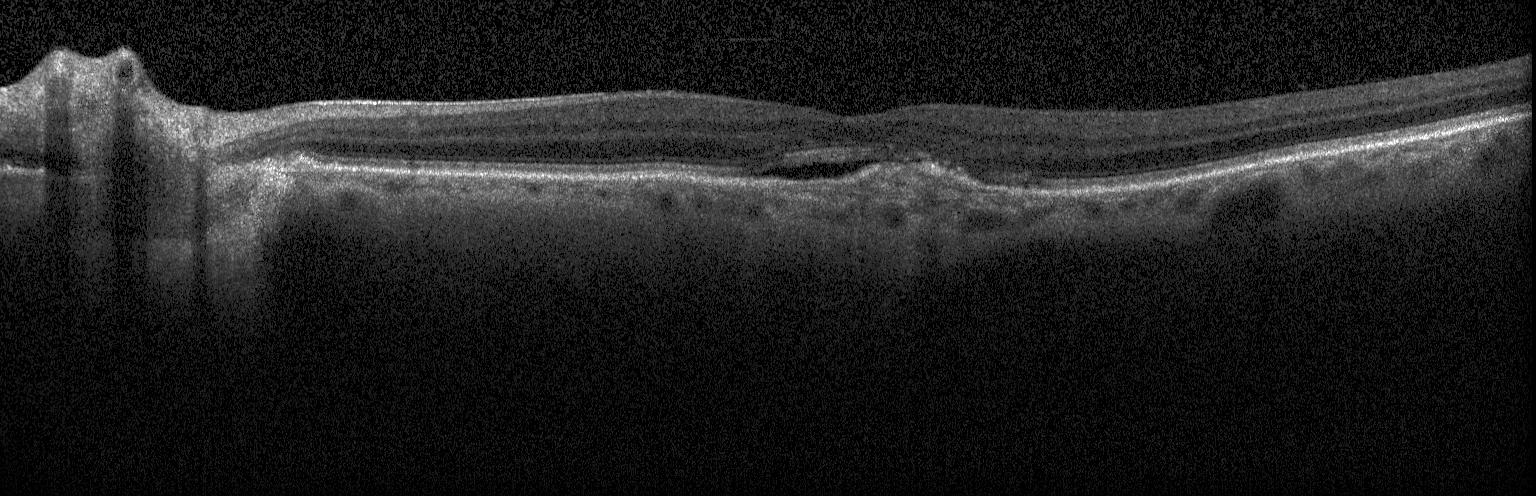

Finding: choroidal neovascularization.